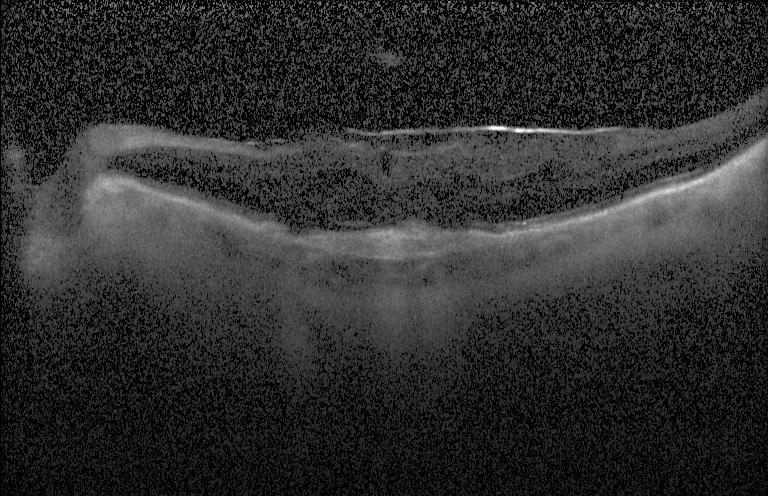 OCT finding: a choroidal neovascular membrane.